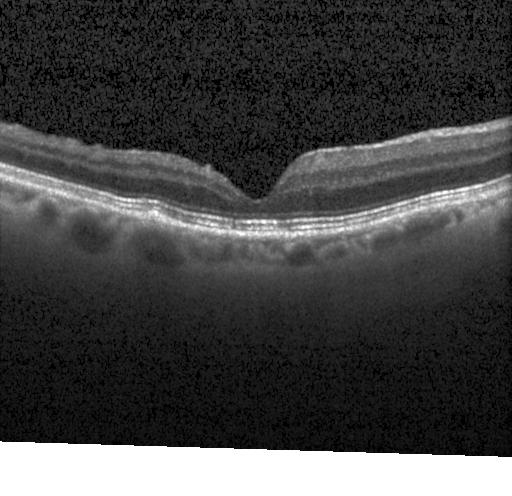 Heidelberg Spectralis OCT system. Spectral-domain OCT. OCT B-scan. Centered on the fovea.
Finding: no choroidal neovascularization, diabetic macular edema, or drusen.